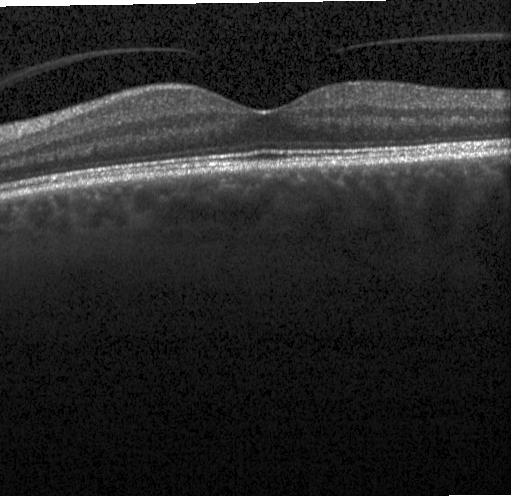

Diagnosis: neither CNV, DME, nor drusen.